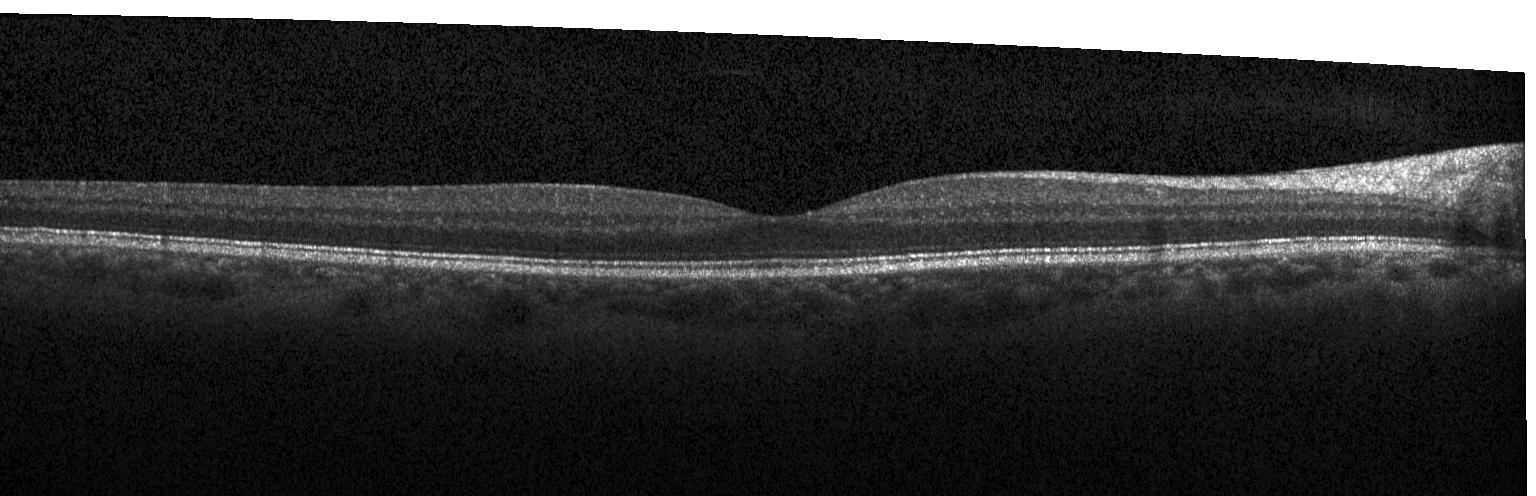

Diagnosis: no choroidal neovascularization, no diabetic macular edema, and no drusen.